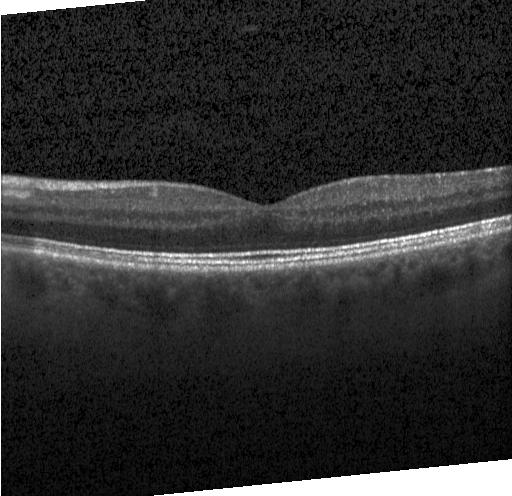

OCT finding: no CNV, DME, or drusen.